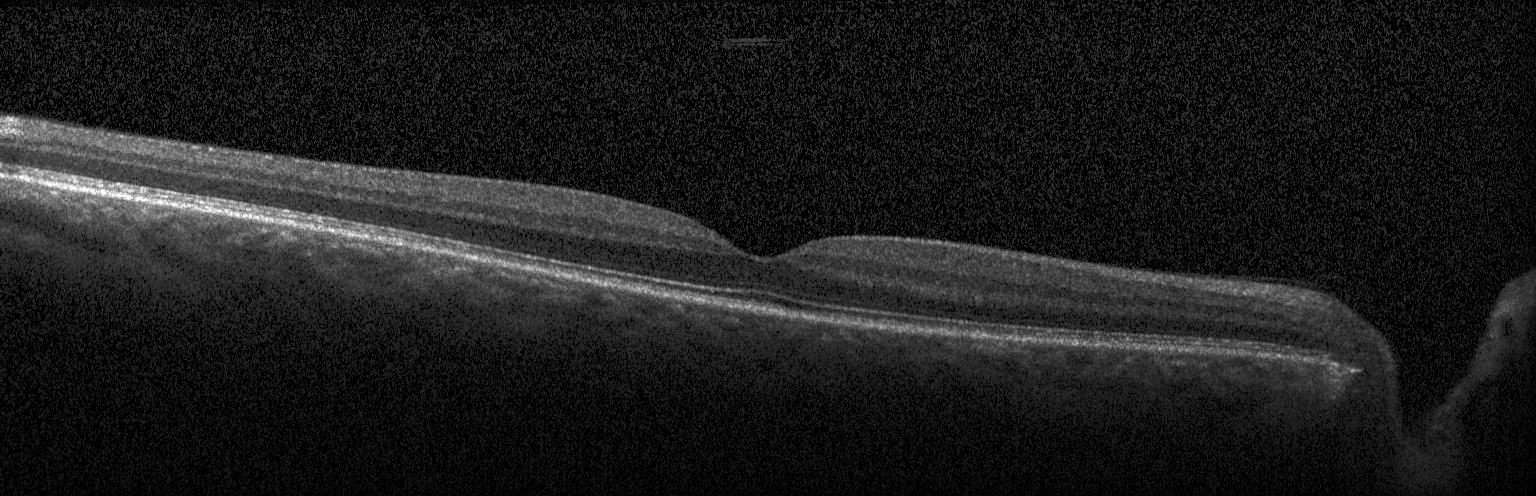 Horizontal scan through the fovea. Optical coherence tomography scan. Heidelberg Spectralis. SD-OCT
OCT finding: no choroidal neovascularization, diabetic macular edema, or drusen.